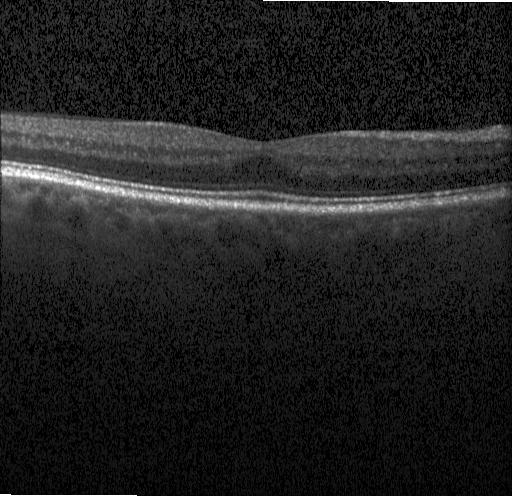

Finding: no CNV, no DME, and no drusen.